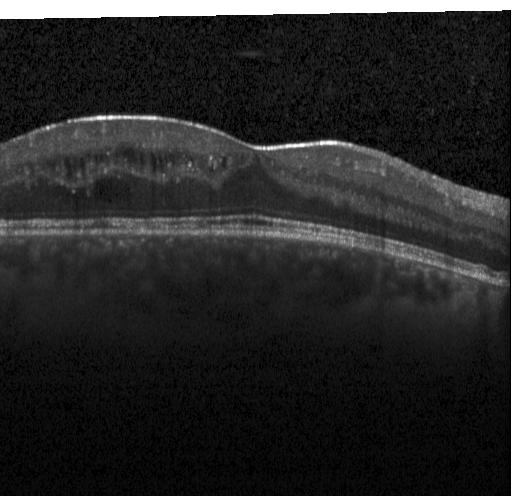
Diagnosis: diabetic macular edema (DME).